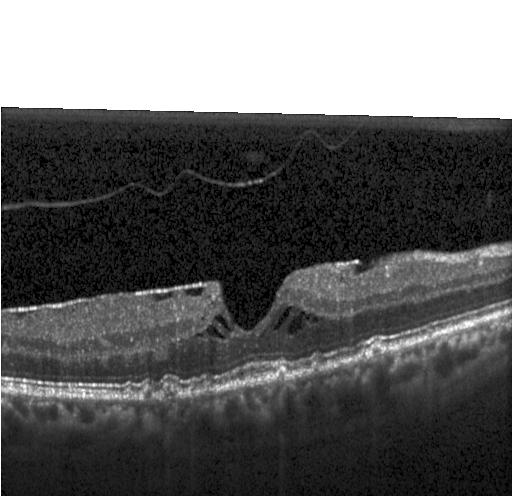
Optical coherence tomography B-scan; instrument: Heidelberg Spectralis; spectral-domain optical coherence tomography
Dx: drusen.